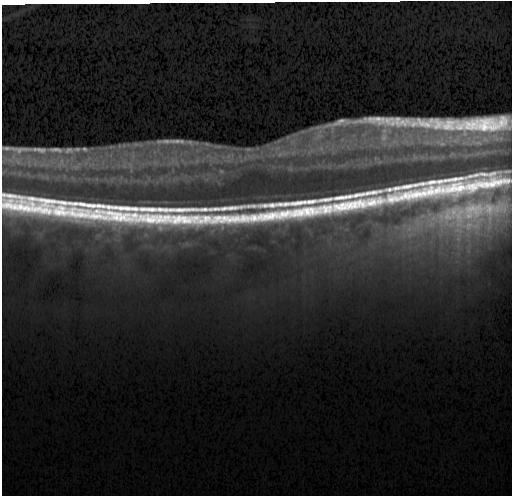
Fovea-centered; spectral-domain OCT; OCT line scan; Heidelberg Spectralis — Impression: no choroidal neovascularization, diabetic macular edema, or drusen.